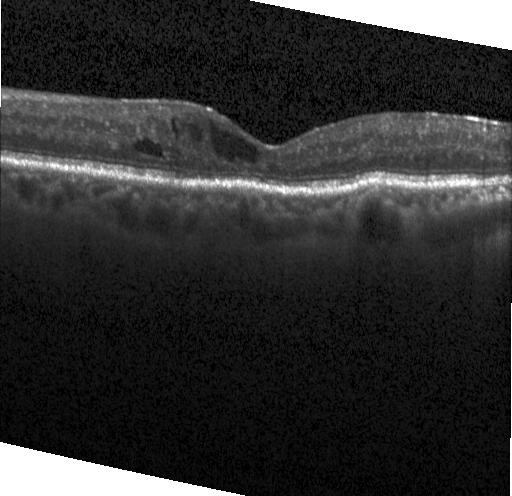

OCT line scan, Heidelberg Spectralis OCT system.
Diabetic macular edema (DME).